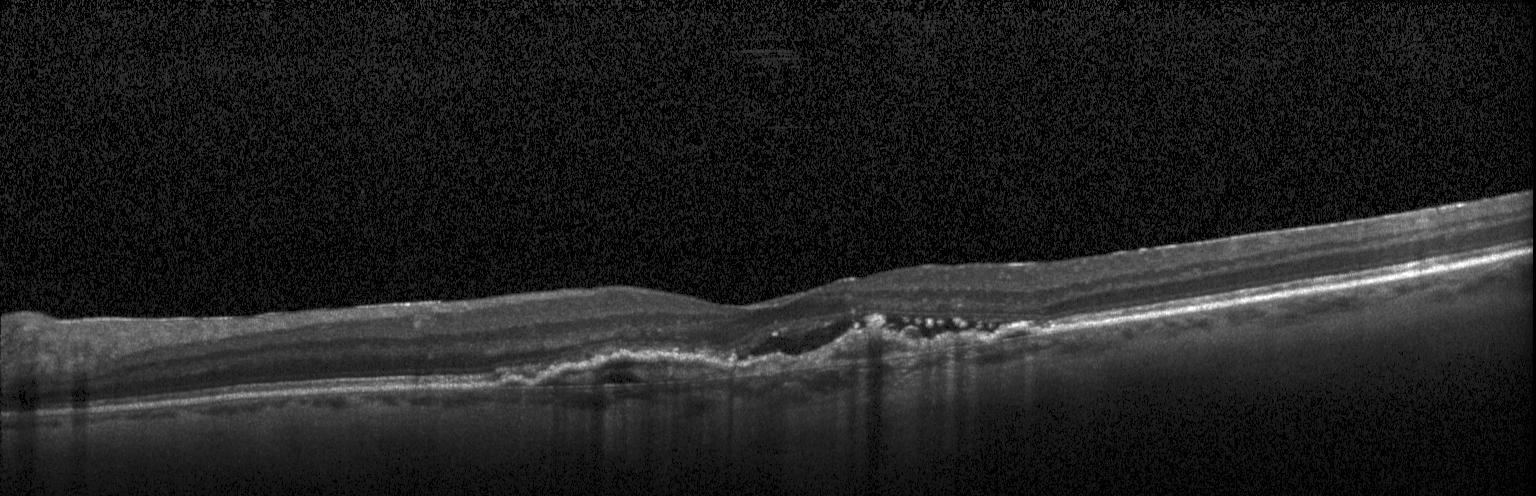 OCT B-scan; fovea-centered. Assessment: CNV.